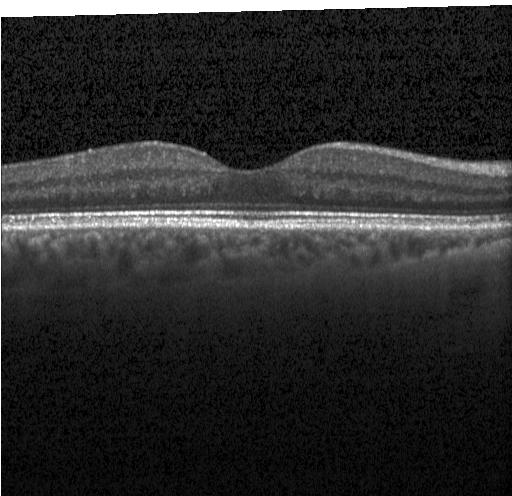

Finding: no evidence of CNV, DME, or drusen.